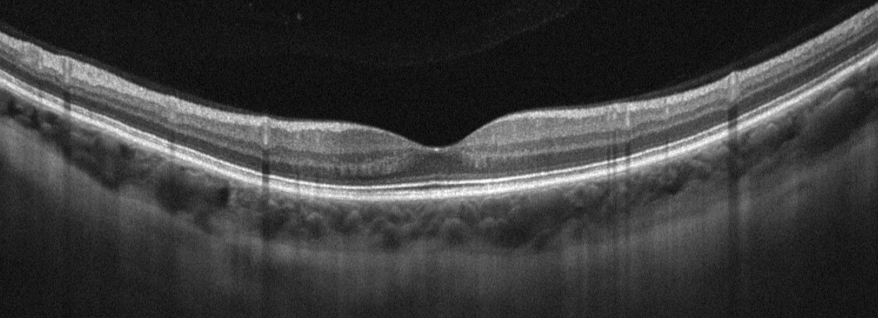
OCT finding: no AMD, DME, ERM, RAO, RVO, or VID.